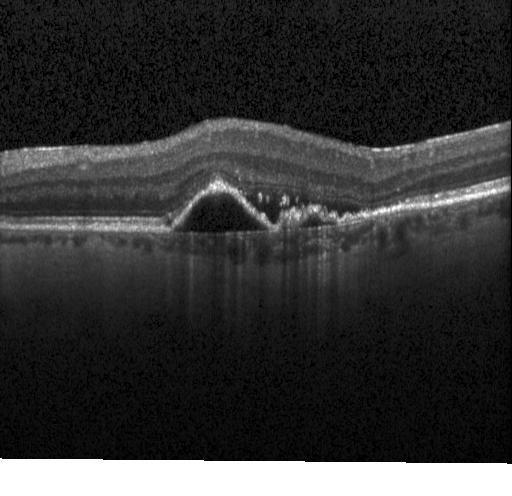

OCT line scan. Spectral-domain OCT. Macular scan.
This B-scan demonstrates choroidal neovascularization.